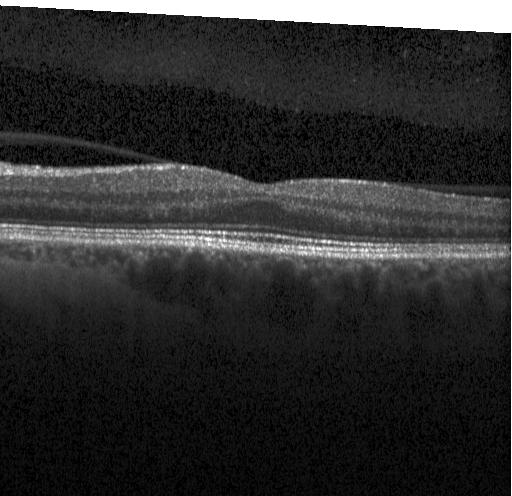

Assessment: no choroidal neovascularization, no diabetic macular edema, and no drusen.